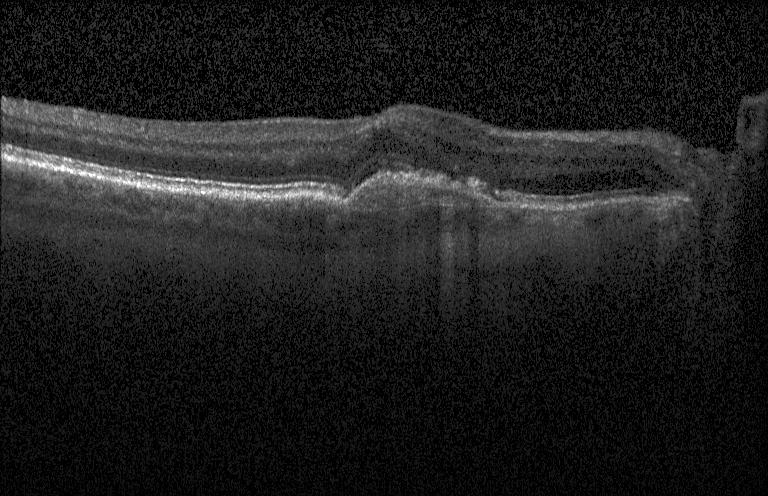

Impression: a choroidal neovascular membrane.